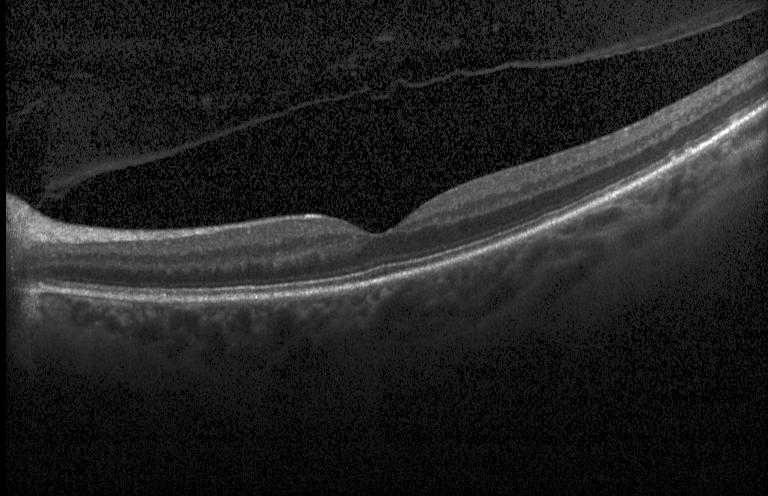

No CNV, no DME, and no drusen.